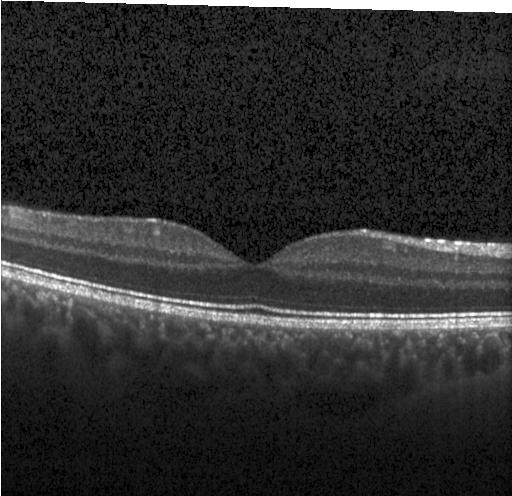 Macular scan · Heidelberg Spectralis OCT system · optical coherence tomography B-scan. Finding: neither choroidal neovascularization, diabetic macular edema, nor drusen.